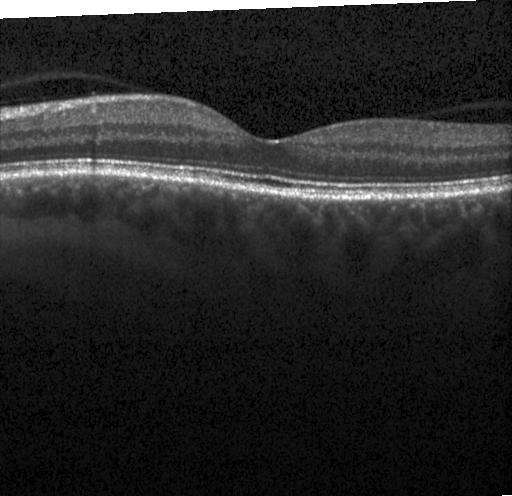
OCT B-scan showing no evidence of CNV, DME, or drusen.